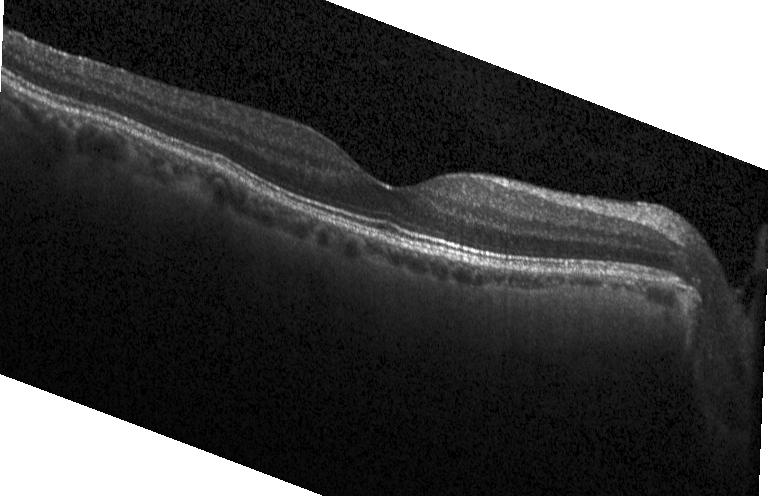
SD-OCT. Retinal OCT cross-section — Impression: no CNV, DME, or drusen.